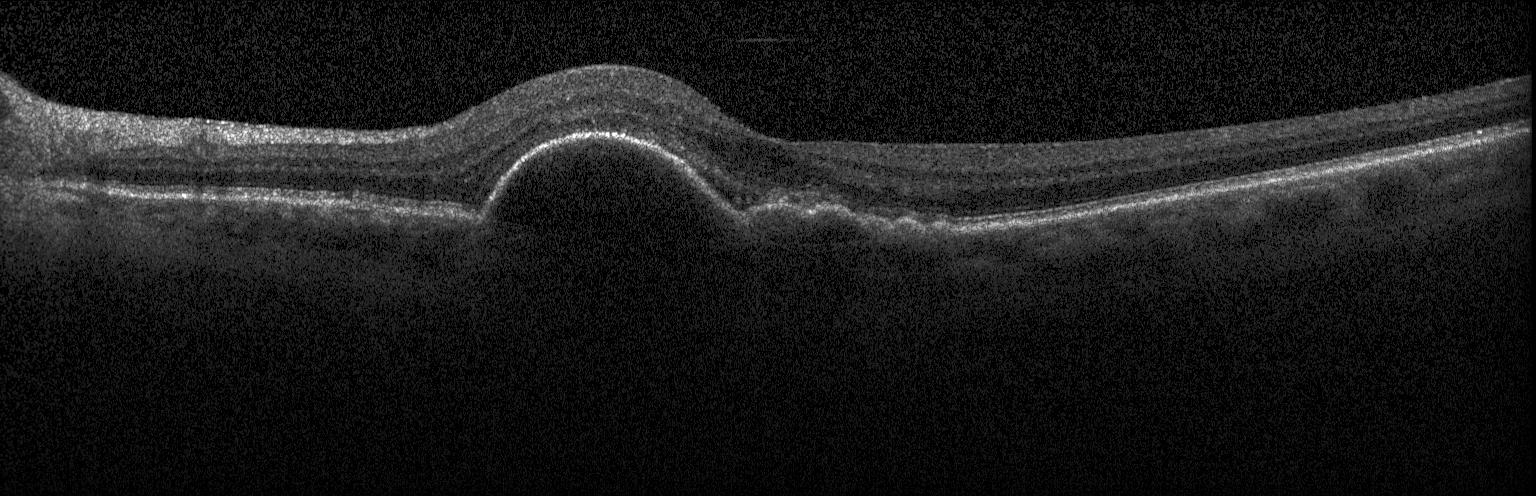

Optical coherence tomography scan. SD-OCT. Macular scan. Heidelberg Spectralis — Dx: a choroidal neovascular membrane.